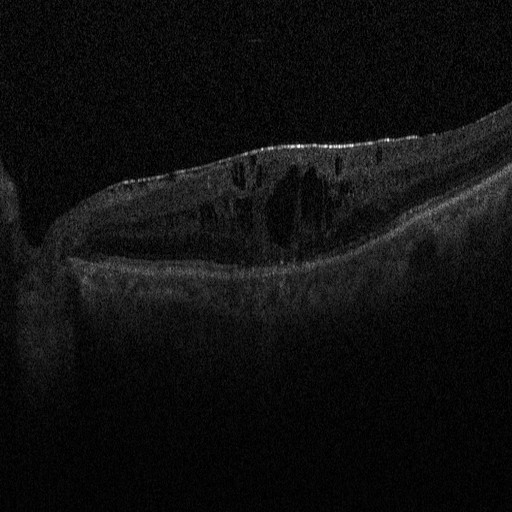 Through the macula; optical coherence tomography B-scan; Heidelberg Spectralis; spectral-domain OCT
Macular OCT: diabetic macular edema (DME).